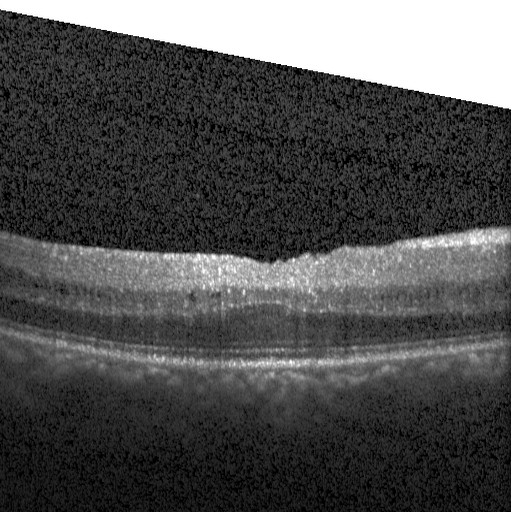
Impression: diabetic macular edema (DME).